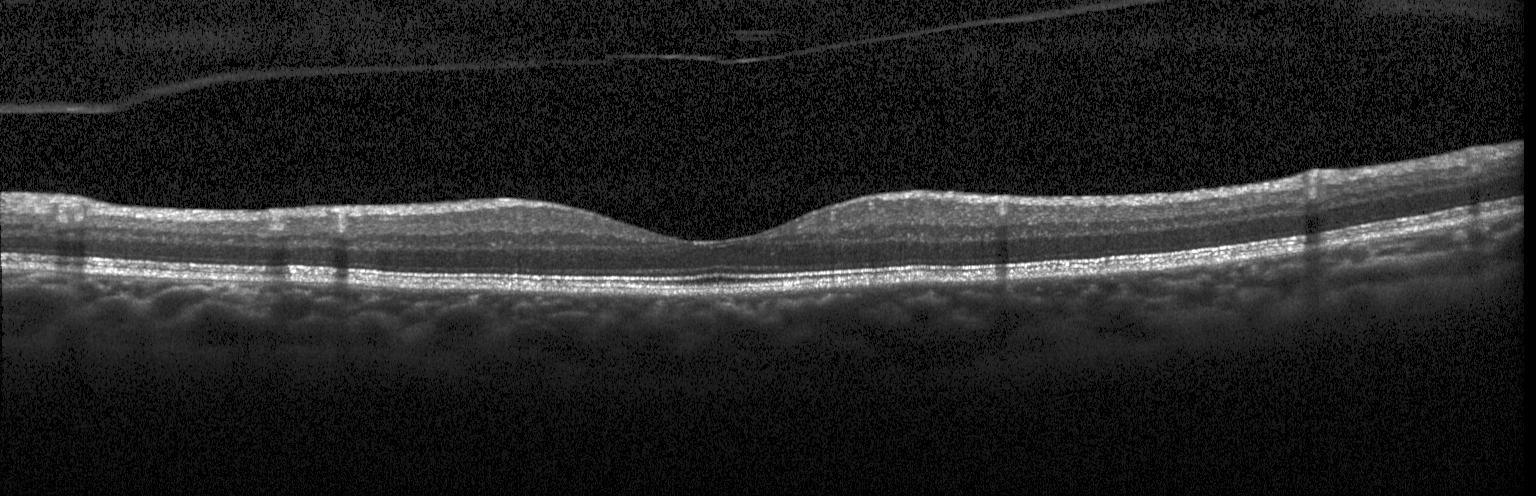 Retinal OCT B-scan. Diagnosis: no evidence of choroidal neovascularization, diabetic macular edema, or drusen.